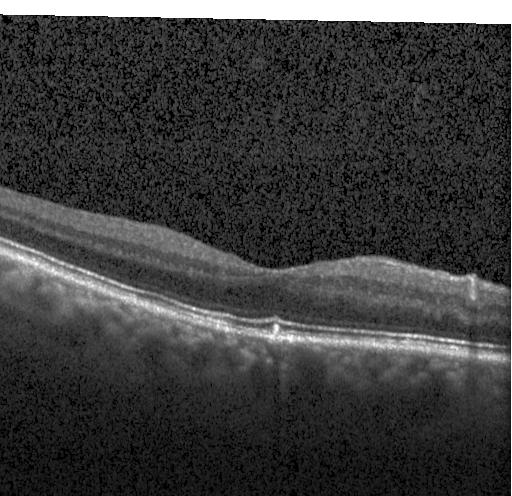 Centered on the fovea. OCT line scan. Instrument: Heidelberg Spectralis
Impression: sub-RPE drusenoid deposits.